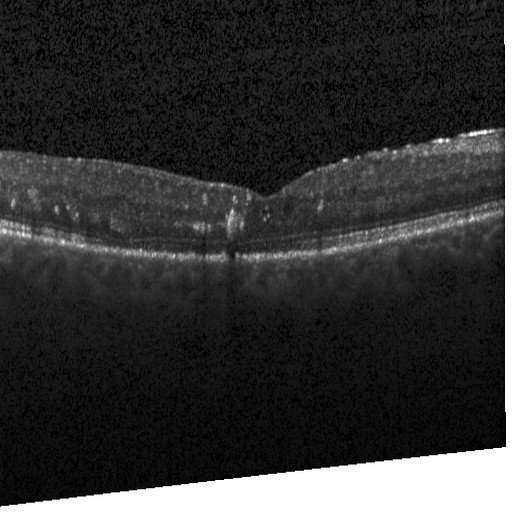

Heidelberg Spectralis OCT system; macular scan; OCT B-scan. Impression: diabetic macular edema.